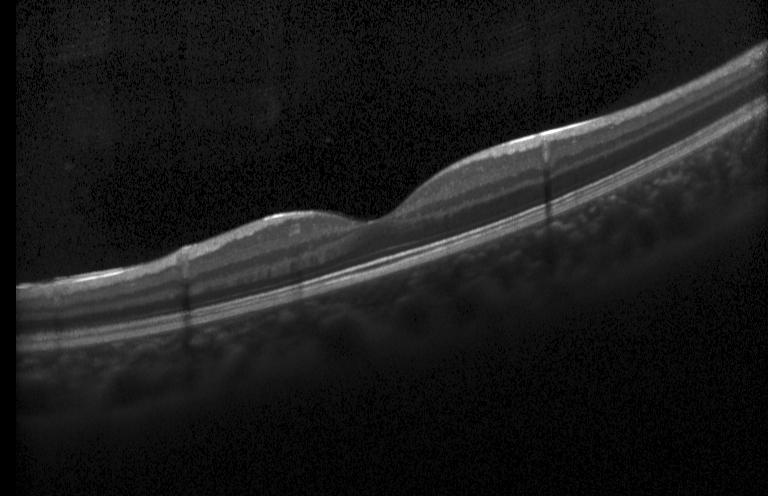
Macular OCT demonstrating neither choroidal neovascularization, diabetic macular edema, nor drusen.